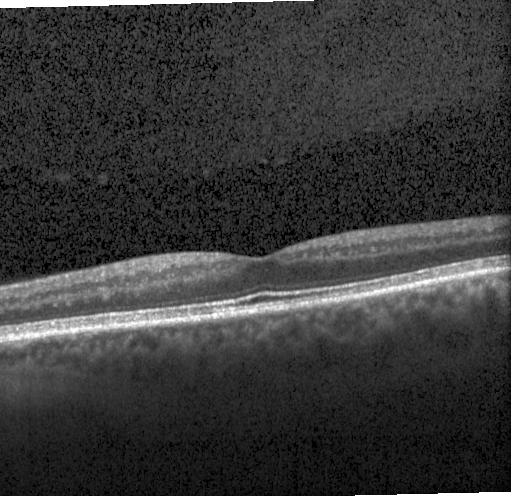

OCT line scan · fovea-centered · SD-OCT · instrument: Heidelberg Spectralis
OCT finding: no choroidal neovascularization, no diabetic macular edema, and no drusen.